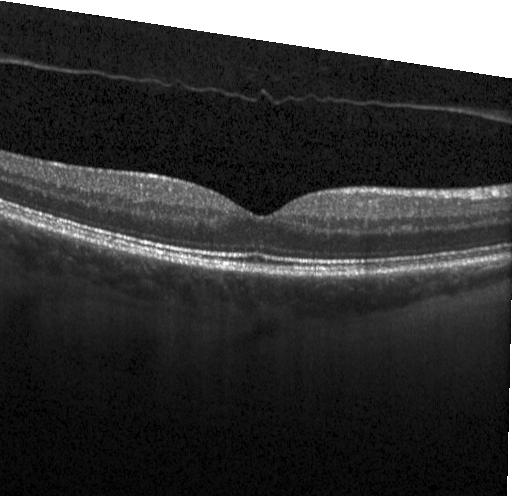

Heidelberg Spectralis. Spectral-domain OCT. Optical coherence tomography B-scan. Macular scan — Macular OCT: no choroidal neovascularization, diabetic macular edema, or drusen.